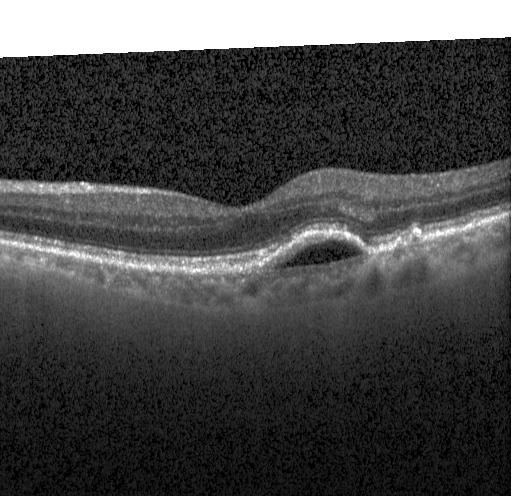 This B-scan demonstrates a choroidal neovascular membrane.